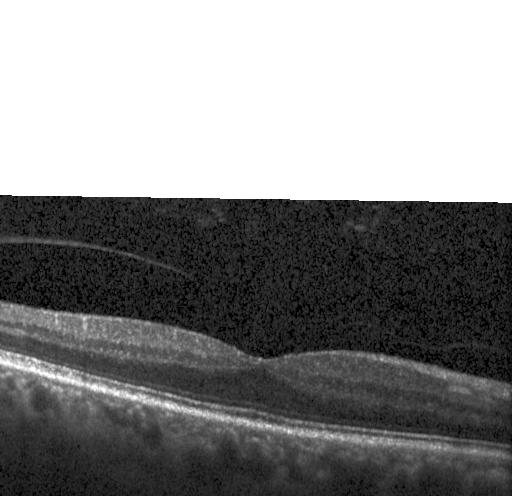

Macular OCT demonstrating no choroidal neovascularization, diabetic macular edema, or drusen.